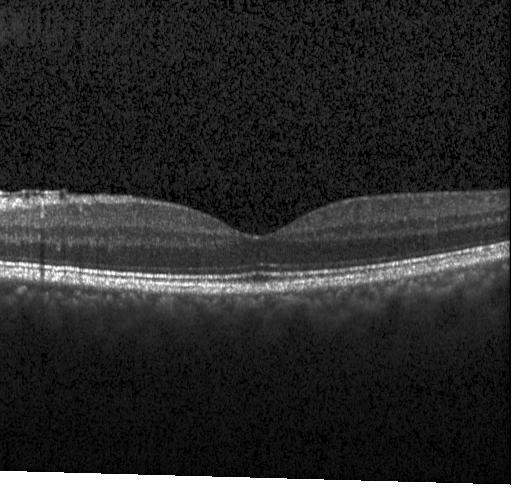
Optical coherence tomography B-scan — Impression: neither choroidal neovascularization, diabetic macular edema, nor drusen.